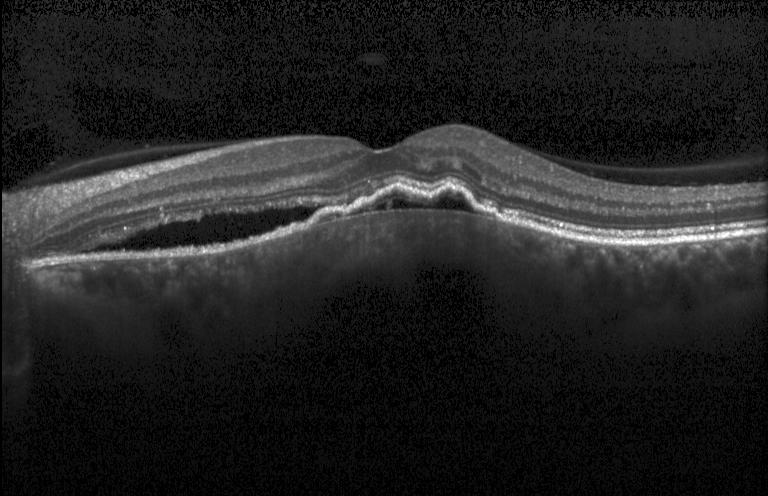
Choroidal neovascularization.